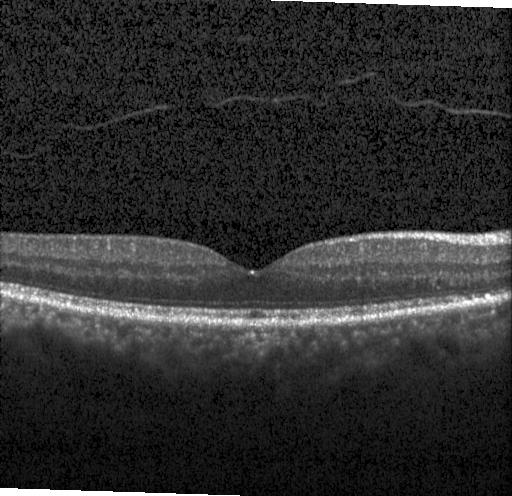 Diagnosis: neither CNV, DME, nor drusen.